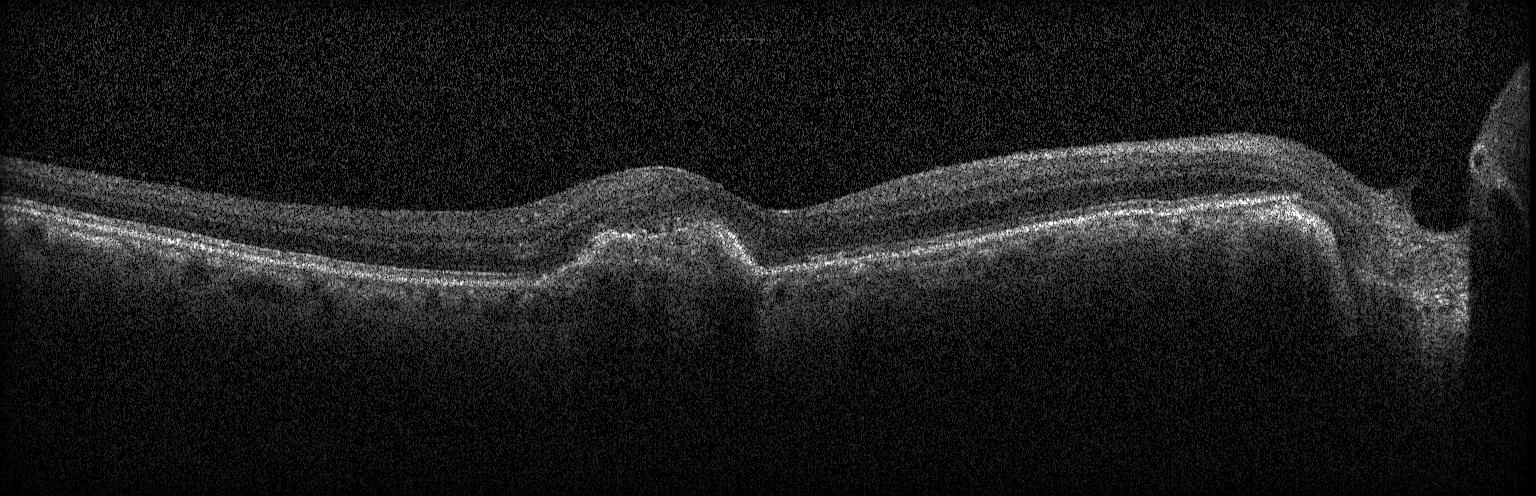
Optical coherence tomography scan. Heidelberg Spectralis.
Diagnosis: choroidal neovascularization.